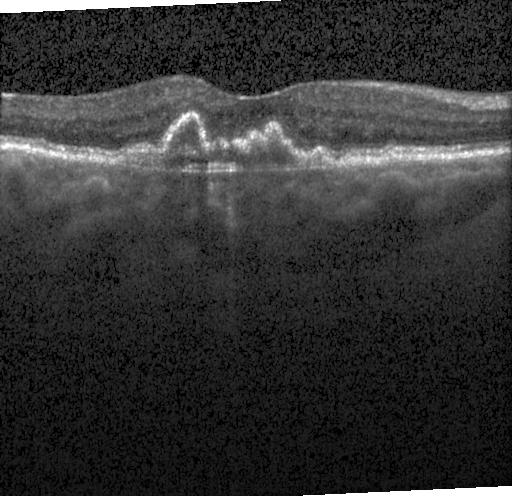
Spectral-domain optical coherence tomography · retinal OCT B-scan · Heidelberg Spectralis OCT system.
Macular OCT: a choroidal neovascular membrane.